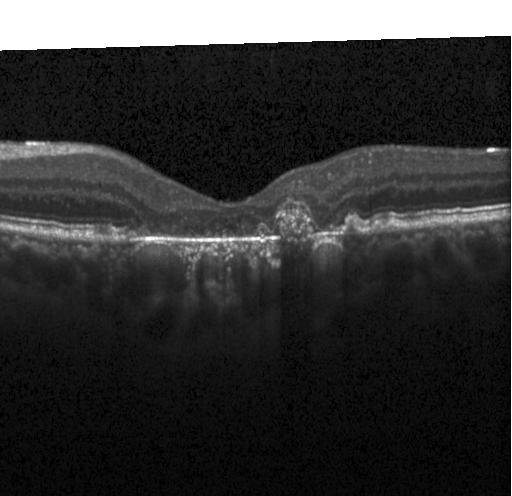
Spectral-domain optical coherence tomography. Retinal OCT B-scan. Macular scan. Heidelberg Spectralis OCT system — Choroidal neovascularization (CNV).